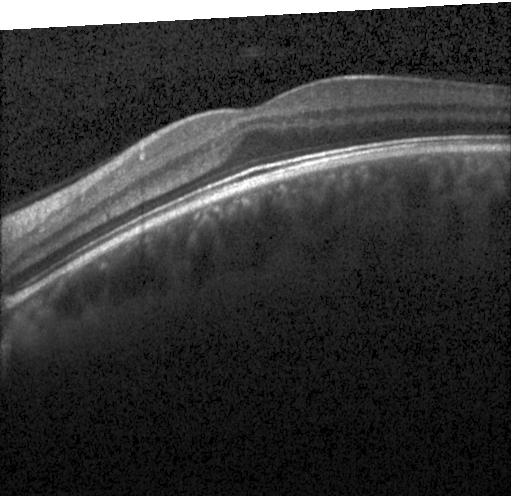
OCT line scan — The scan shows no evidence of choroidal neovascularization, diabetic macular edema, or drusen.